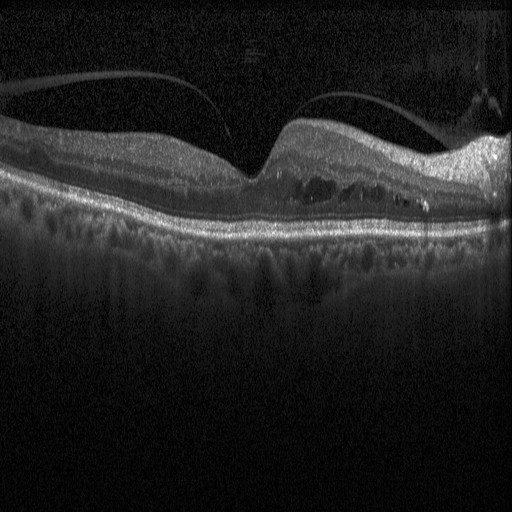 Retinal OCT B-scan
Impression: diabetic macular edema.